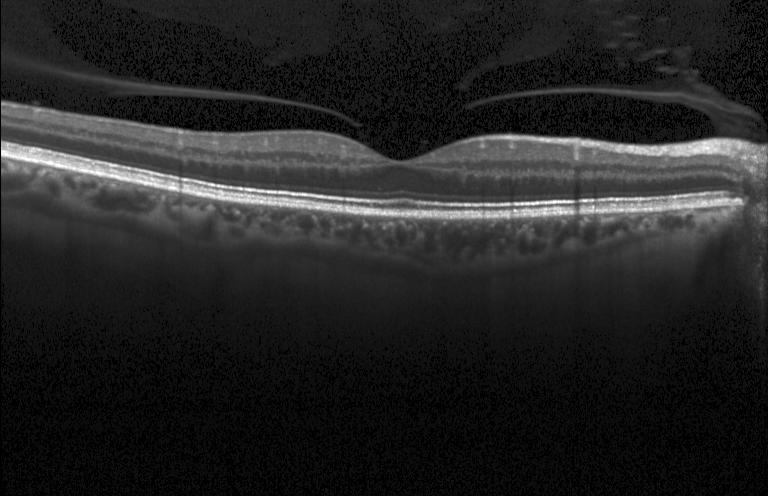 Macular OCT demonstrating neither CNV, DME, nor drusen.